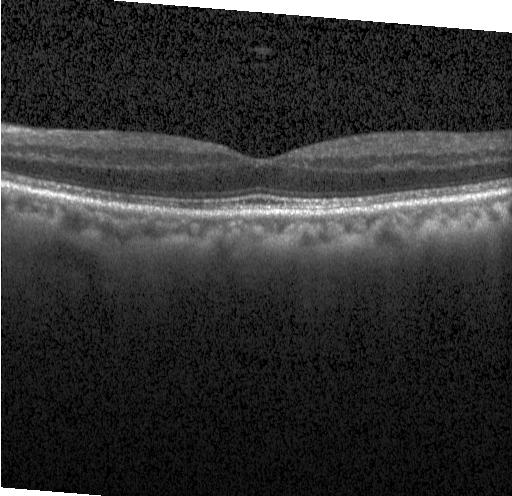 OCT B-scan showing no CNV, DME, or drusen.